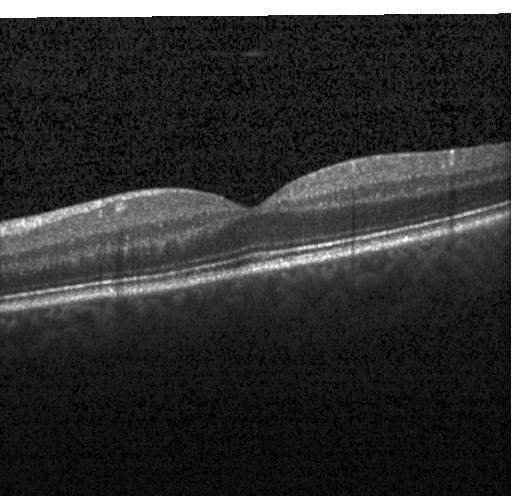
Macular scan. SD-OCT. Optical coherence tomography scan. Heidelberg Spectralis — Impression: no choroidal neovascularization, diabetic macular edema, or drusen.